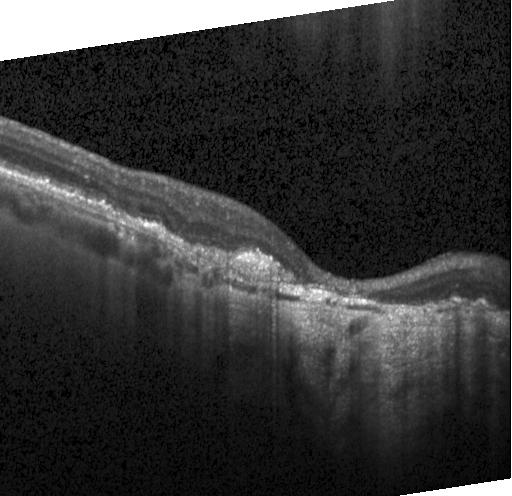
Dx: a choroidal neovascular membrane.